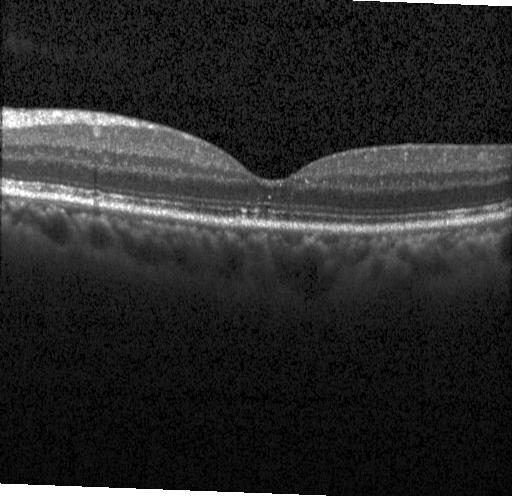
Heidelberg Spectralis; retinal OCT cross-section; spectral-domain OCT.
The scan shows no choroidal neovascularization, no diabetic macular edema, and no drusen.